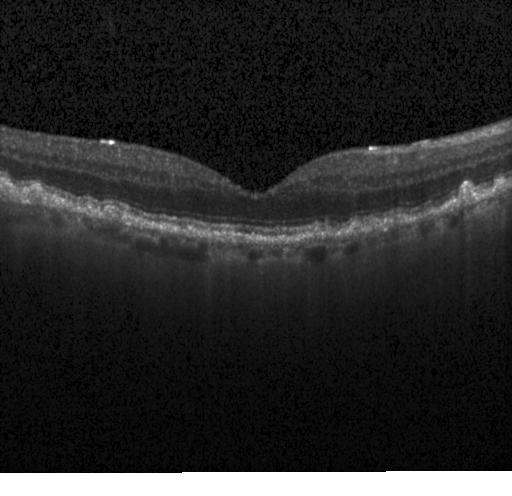

Macular scan. Heidelberg Spectralis OCT system. Retinal OCT cross-section — This B-scan demonstrates sub-RPE drusenoid deposits.